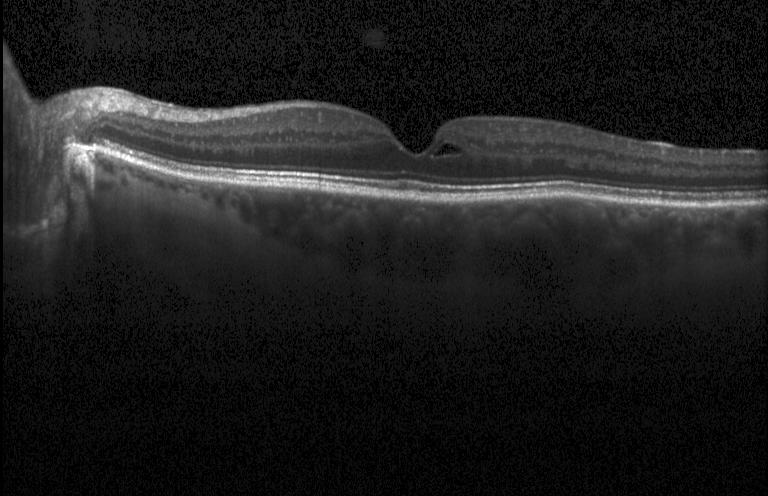

Optical coherence tomography scan, spectral-domain OCT
DME.